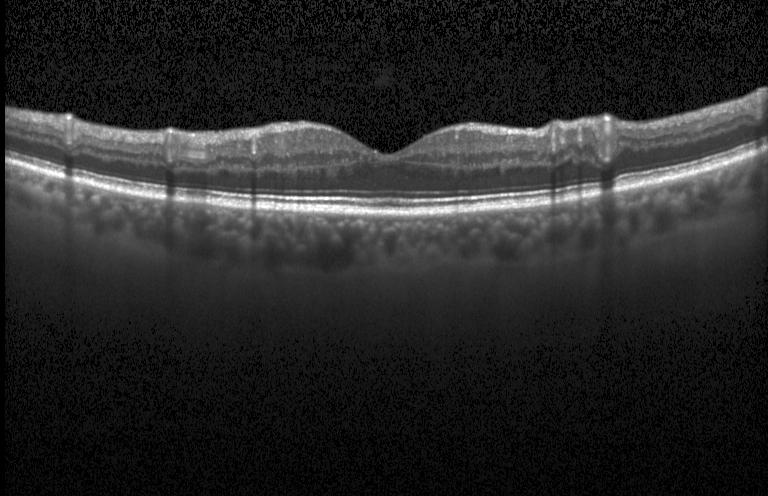

Macular OCT: no CNV, no DME, and no drusen.